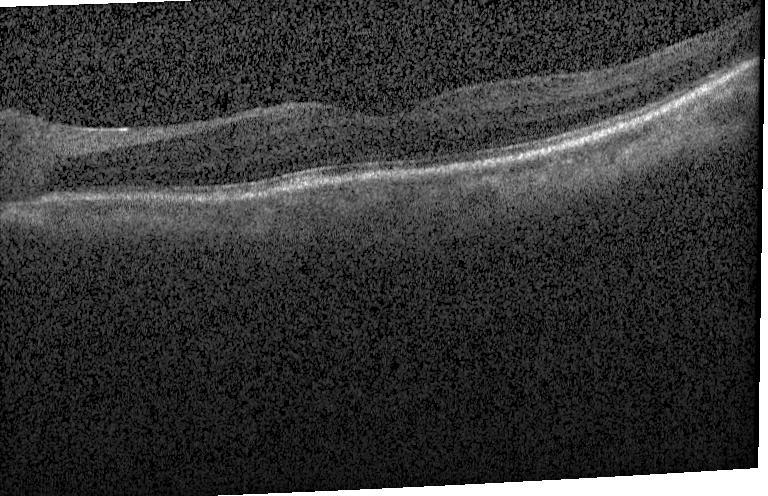 Horizontal scan through the fovea · OCT line scan · SD-OCT · acquired on a Heidelberg Spectralis. This B-scan demonstrates no CNV, no DME, and no drusen.